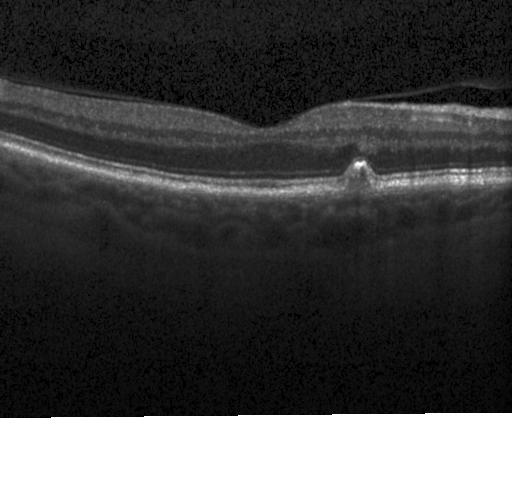
SD-OCT · optical coherence tomography scan
Sub-RPE drusenoid deposits.